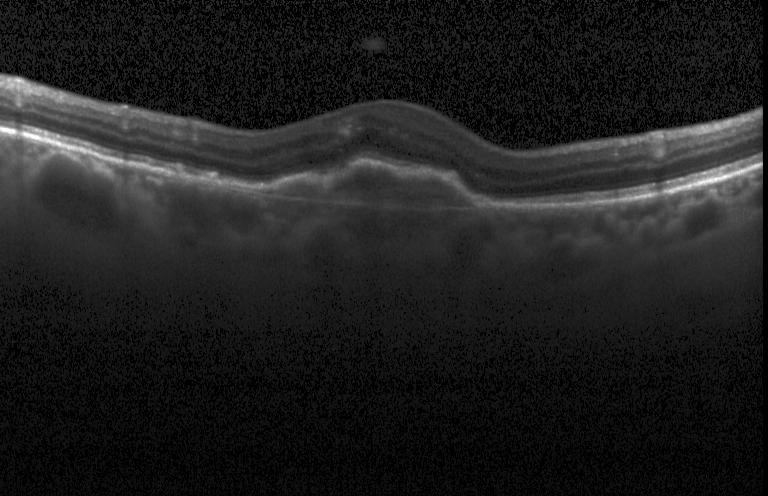
Diagnosis: choroidal neovascularization.